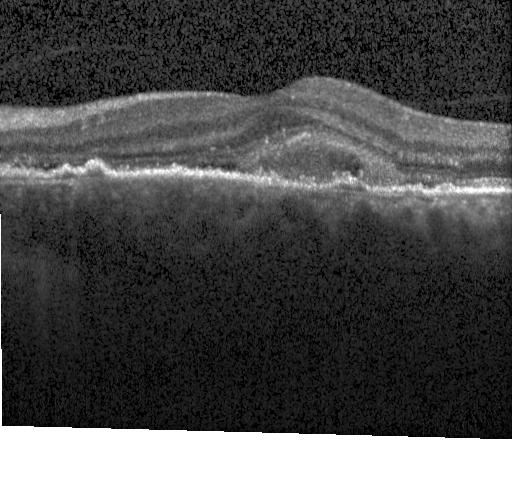
Choroidal neovascularization (CNV).